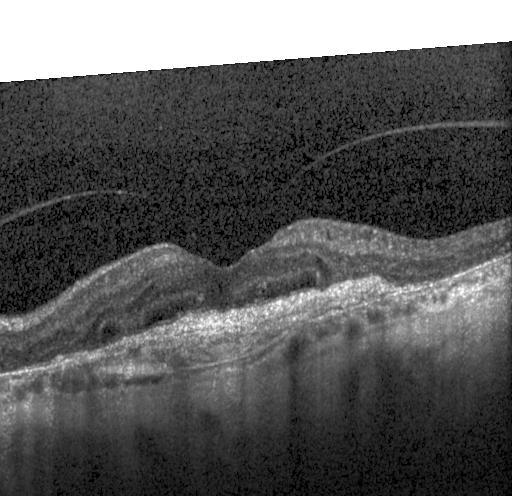
This B-scan demonstrates choroidal neovascularization.